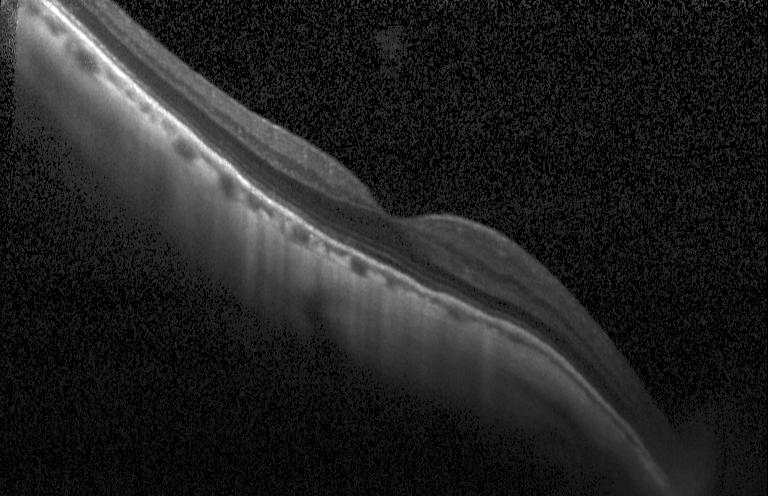 Instrument: Heidelberg Spectralis; OCT B-scan; spectral-domain optical coherence tomography.
Macular OCT: no choroidal neovascularization, diabetic macular edema, or drusen.